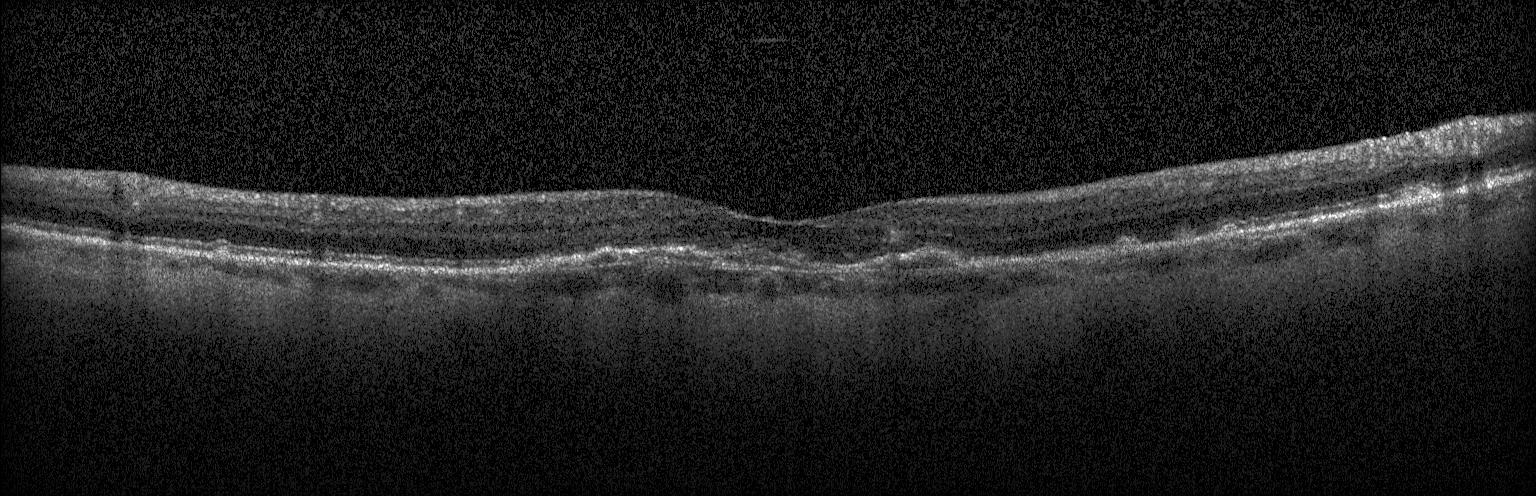 OCT line scan · instrument: Heidelberg Spectralis · horizontal scan through the fovea.
Impression: a choroidal neovascular membrane.